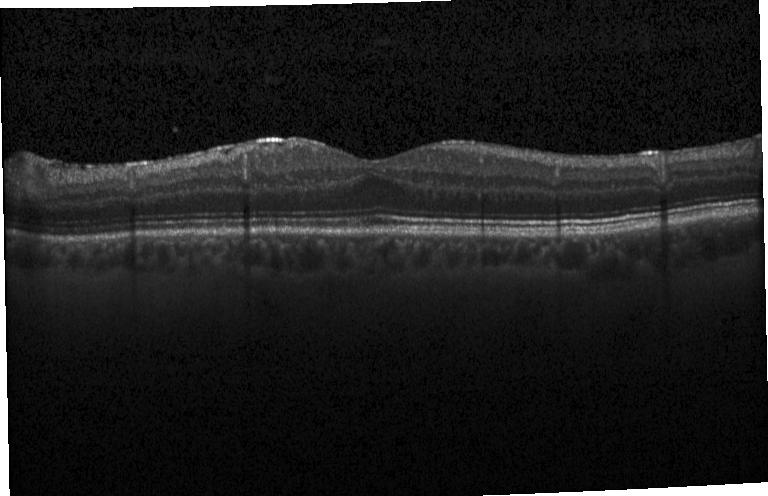
OCT B-scan, horizontal scan through the fovea, Heidelberg Spectralis OCT system.
Finding: no CNV, DME, or drusen.